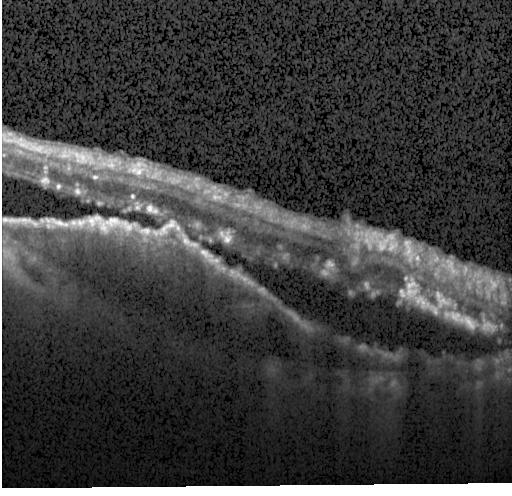
Macular scan · OCT B-scan · spectral-domain OCT · instrument: Heidelberg Spectralis — Finding: CNV.